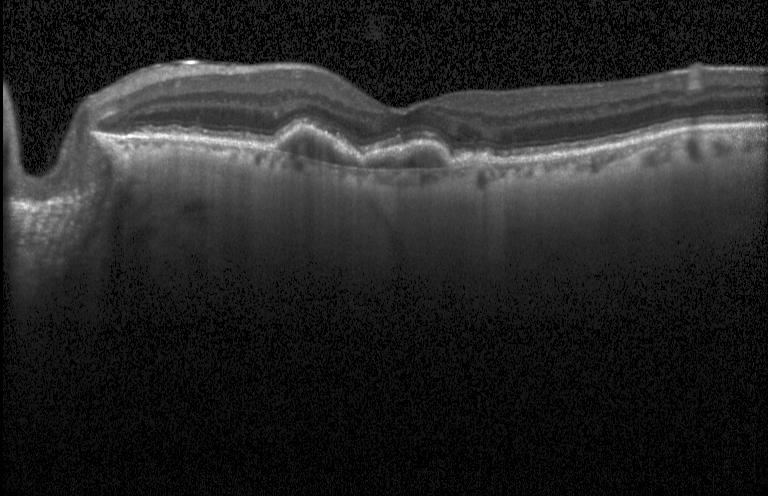
This B-scan demonstrates a choroidal neovascular membrane.